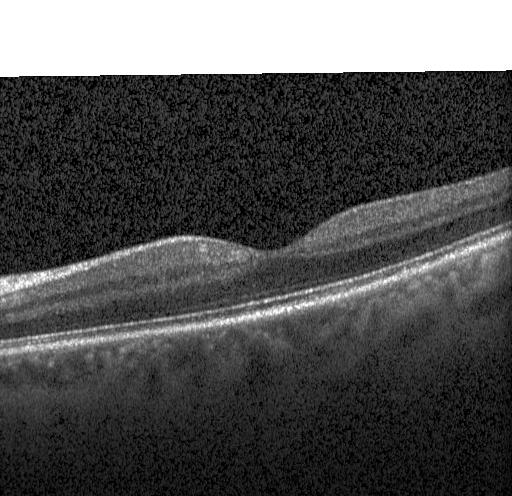

The scan shows no CNV, no DME, and no drusen.